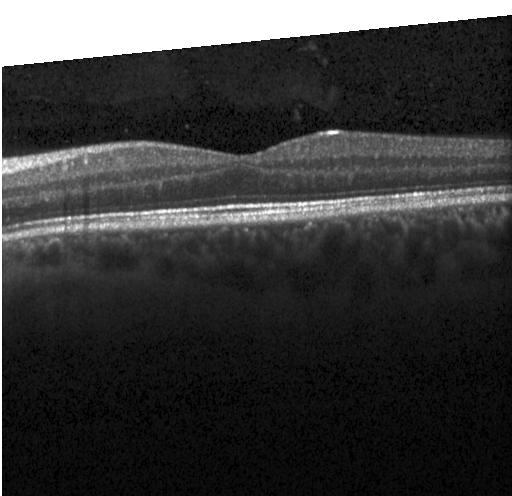

OCT B-scan. Impression: no CNV, no DME, and no drusen.